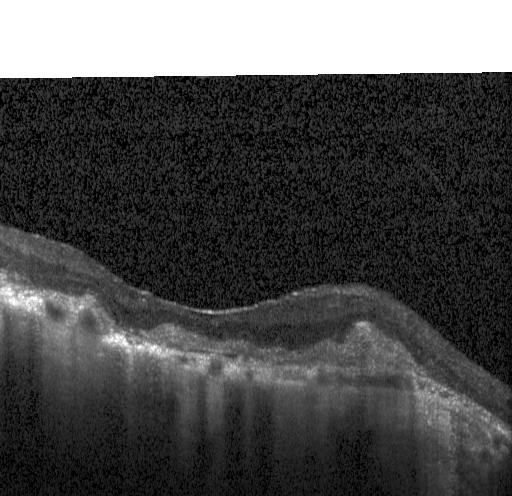 Heidelberg Spectralis OCT system · OCT line scan.
This B-scan demonstrates a choroidal neovascular membrane.